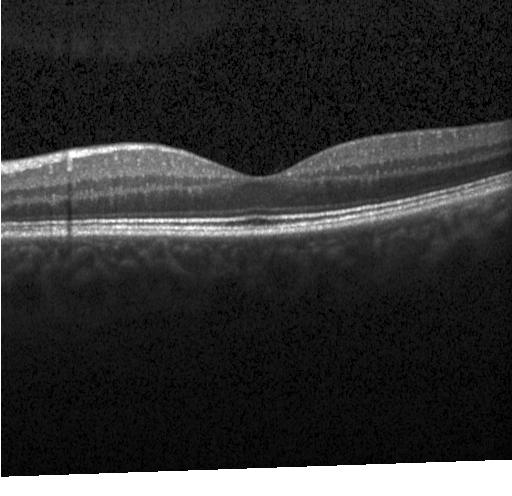
Diagnosis: neither CNV, DME, nor drusen.